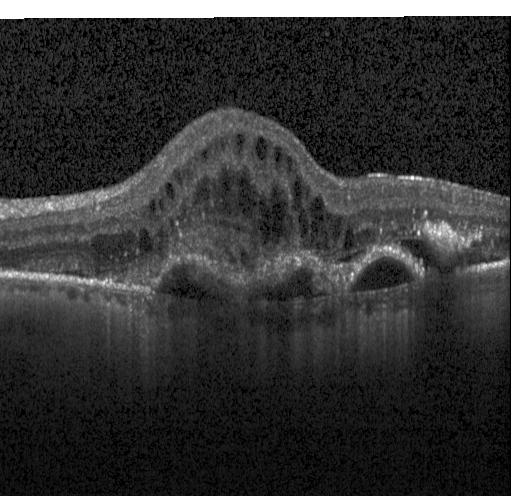 Finding: choroidal neovascularization (CNV).